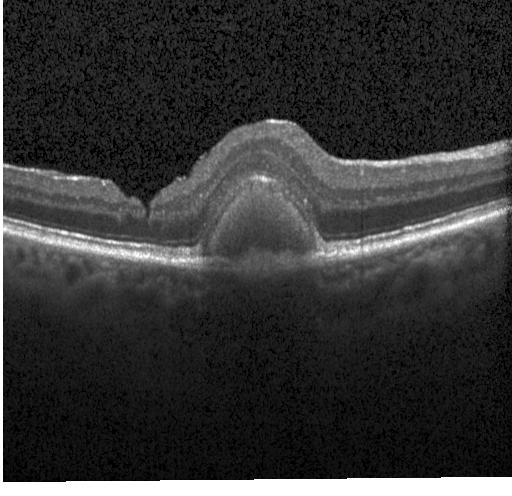

Impression: CNV.